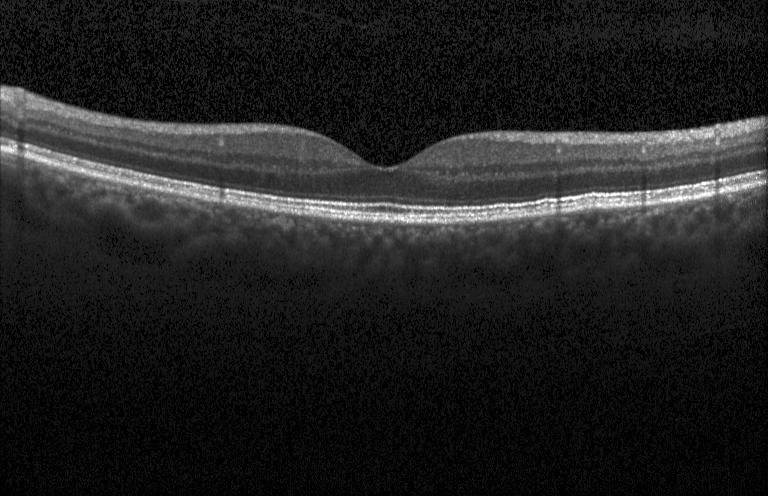

Finding: no CNV, DME, or drusen.